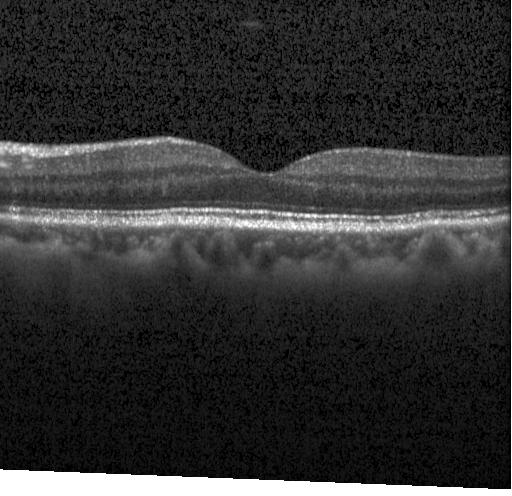 Spectral-domain OCT · optical coherence tomography scan · Heidelberg Spectralis. No choroidal neovascularization, diabetic macular edema, or drusen.